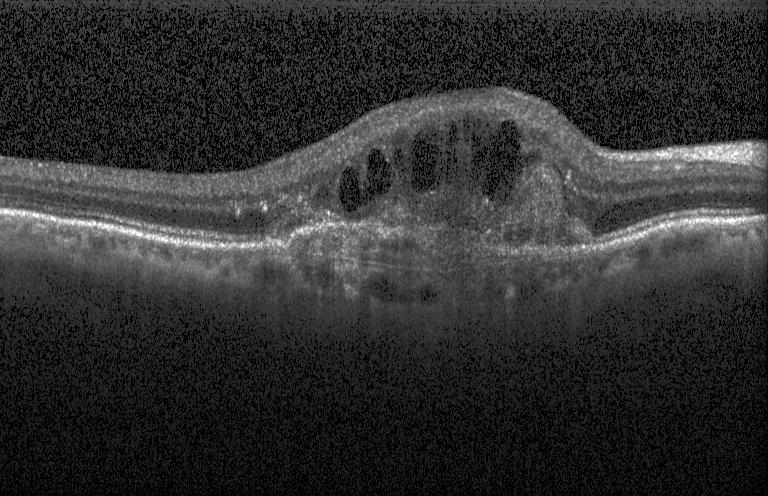

Finding: choroidal neovascularization.